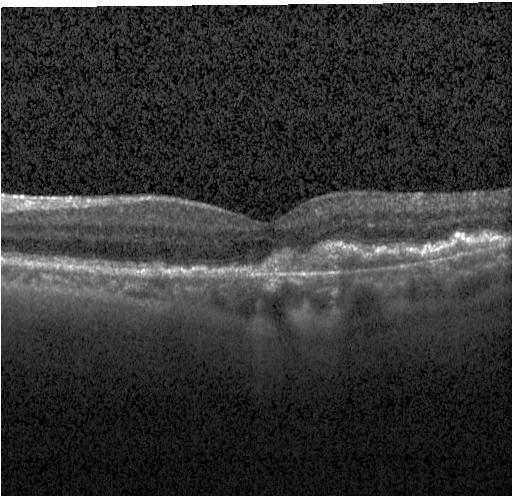
Diagnosis: choroidal neovascularization.